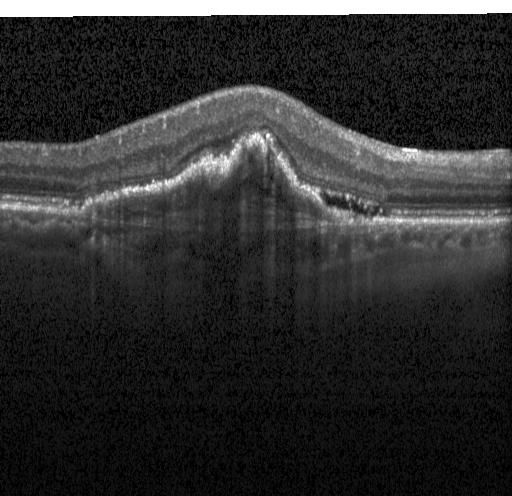
Macular OCT demonstrating a choroidal neovascular membrane.